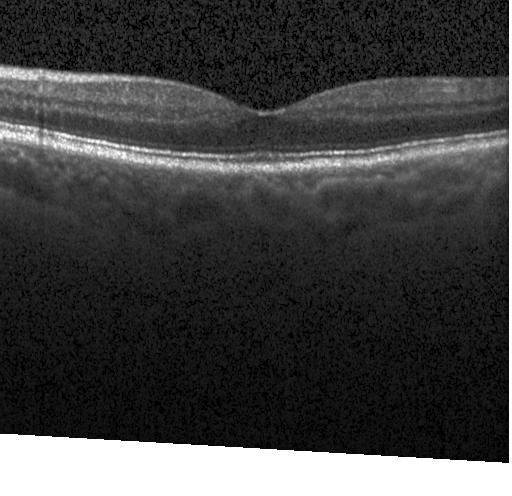
Spectral-domain OCT B-scan: no choroidal neovascularization, no diabetic macular edema, and no drusen.